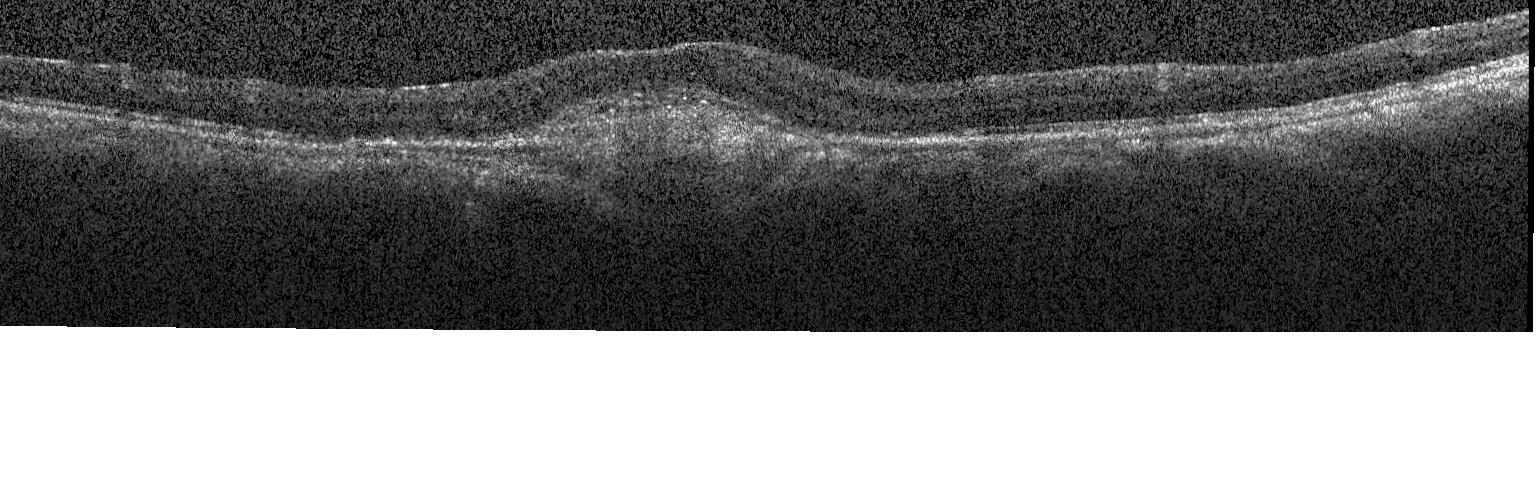

OCT B-scan. Choroidal neovascularization (CNV).